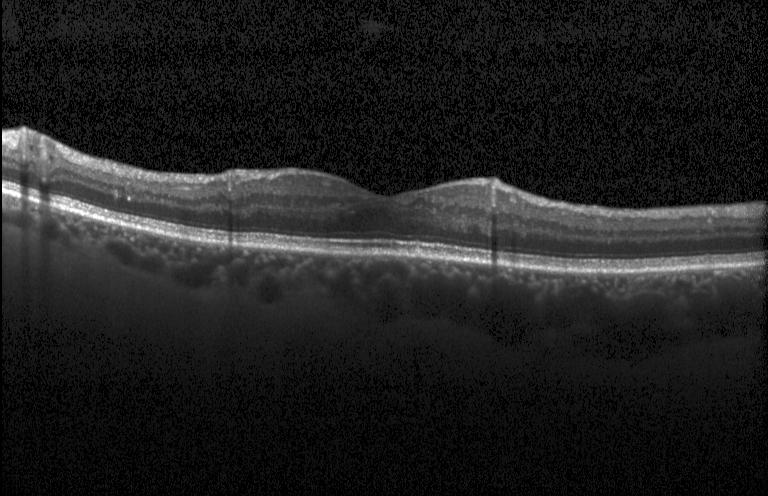 Instrument: Heidelberg Spectralis, spectral-domain OCT, OCT line scan, fovea-centered — Finding: no choroidal neovascularization, no diabetic macular edema, and no drusen.